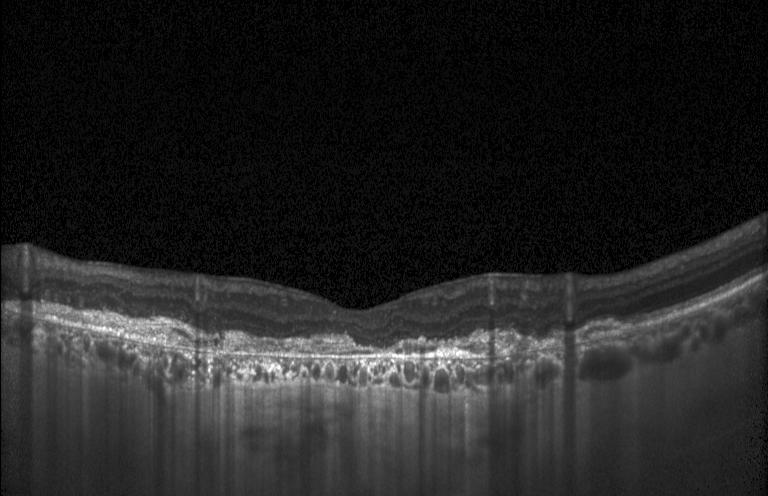
OCT B-scan showing a choroidal neovascular membrane.